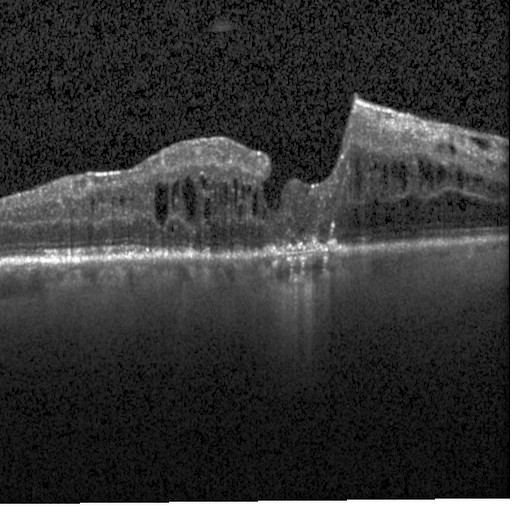

Heidelberg Spectralis OCT system, optical coherence tomography scan, fovea-centered — Diagnosis: diabetic macular edema (DME).